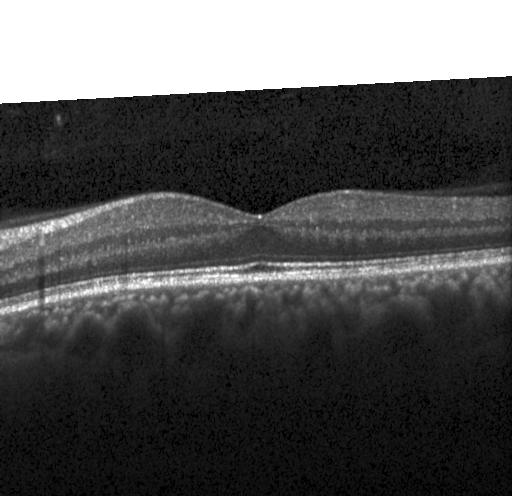 Optical coherence tomography scan; acquired on a Heidelberg Spectralis; spectral-domain optical coherence tomography — Macular OCT: neither CNV, DME, nor drusen.